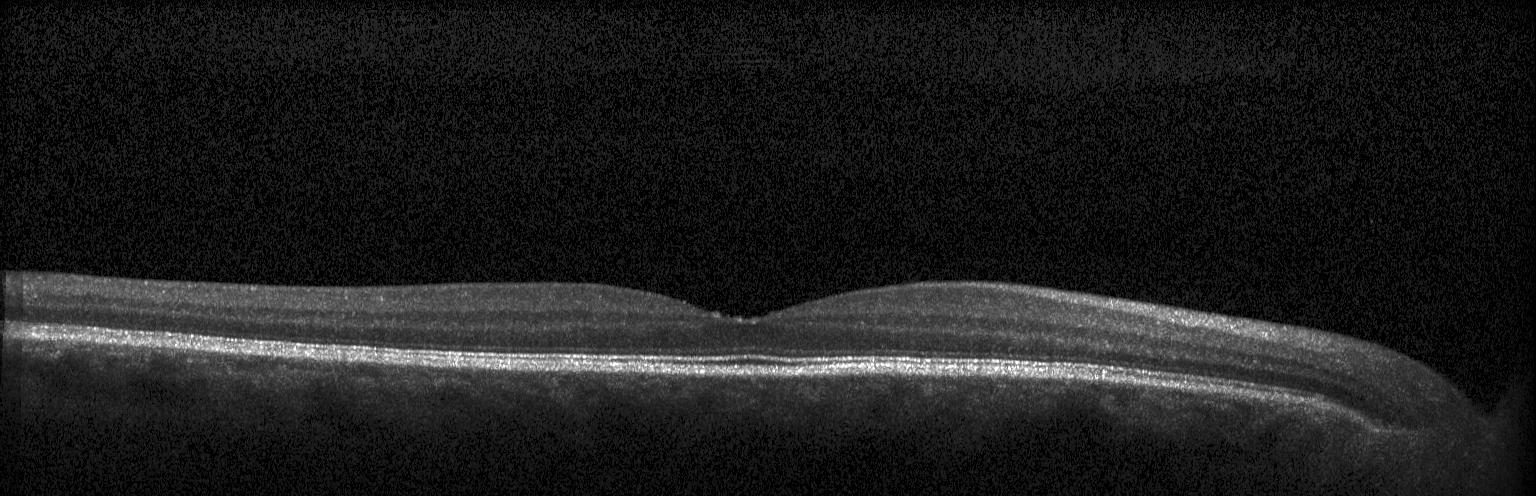

Optical coherence tomography scan, spectral-domain OCT — The scan shows no evidence of choroidal neovascularization, diabetic macular edema, or drusen.